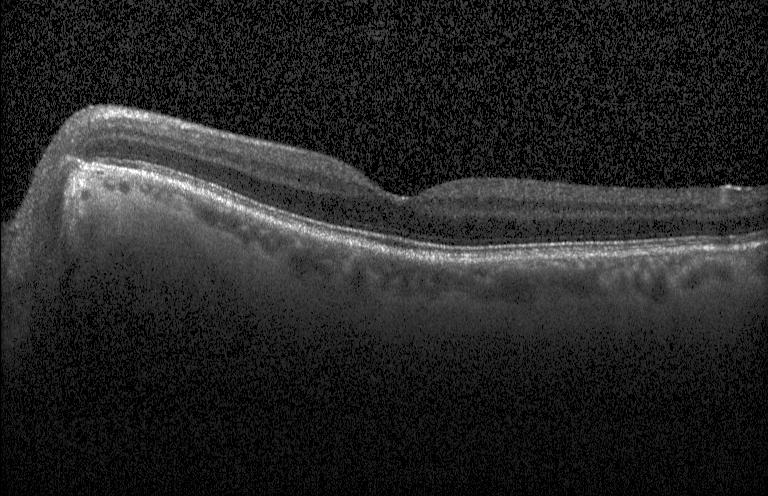
Optical coherence tomography scan · spectral-domain optical coherence tomography. Impression: no evidence of CNV, DME, or drusen.